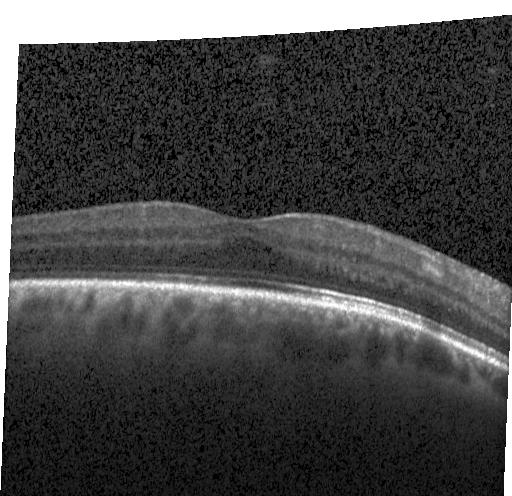 Retinal OCT B-scan; fovea-centered.
Impression: no CNV, no DME, and no drusen.